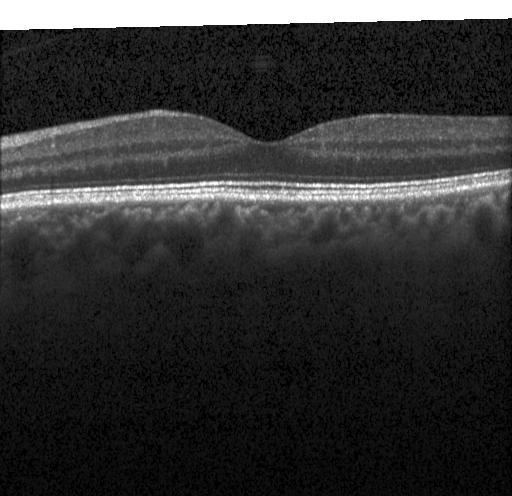

Optical coherence tomography scan; spectral-domain OCT — The scan shows neither CNV, DME, nor drusen.